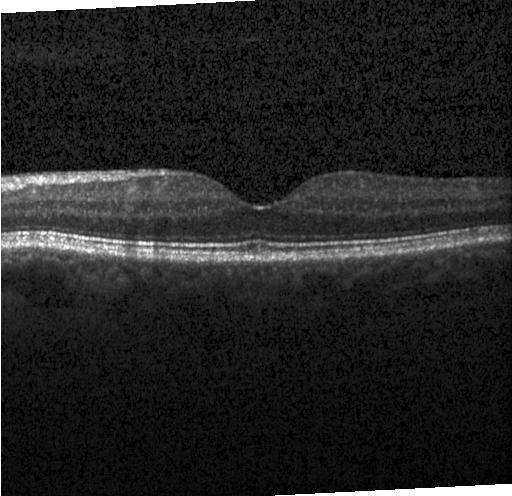

Finding: no evidence of CNV, DME, or drusen.